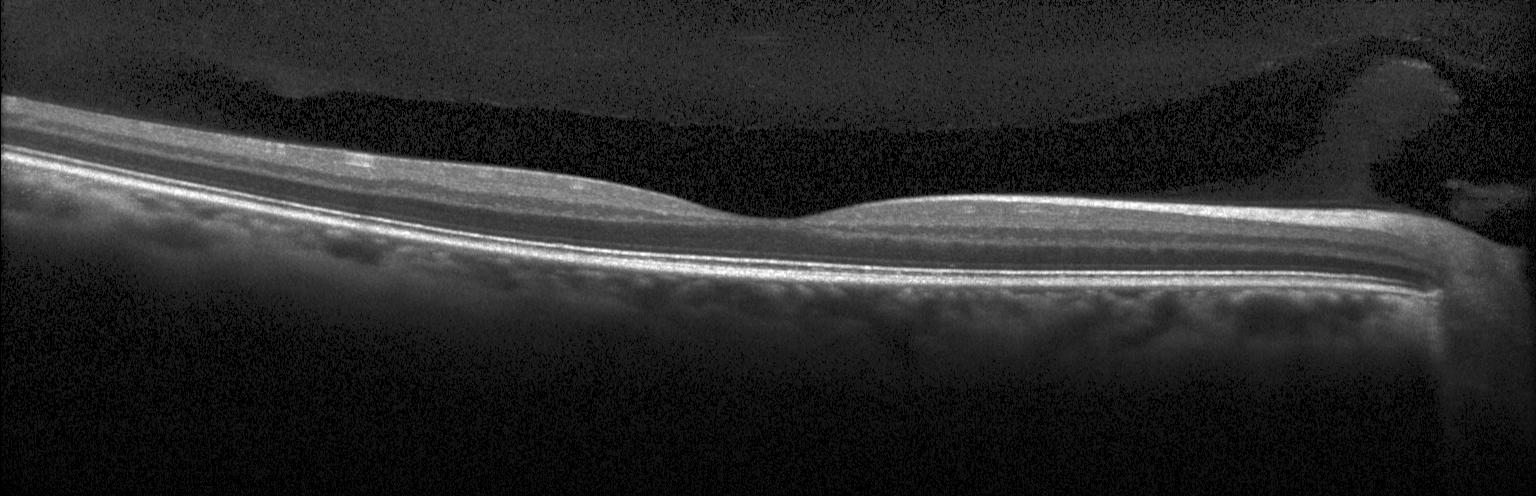 Retinal OCT B-scan. Neither choroidal neovascularization, diabetic macular edema, nor drusen.